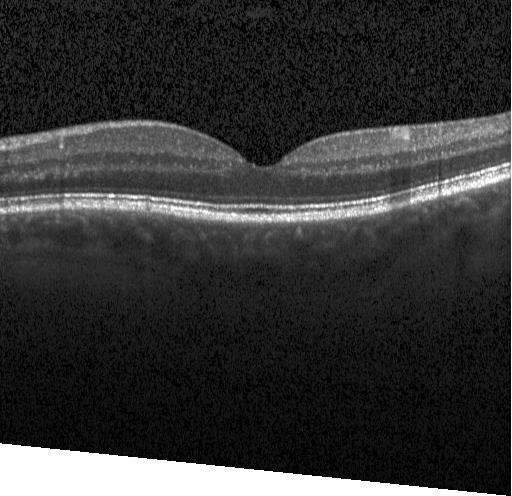

Retinal OCT cross-section showing neither choroidal neovascularization, diabetic macular edema, nor drusen.